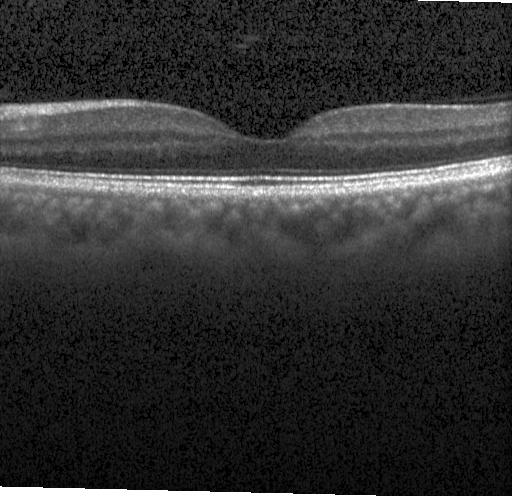
OCT line scan · Heidelberg Spectralis — Neither choroidal neovascularization, diabetic macular edema, nor drusen.